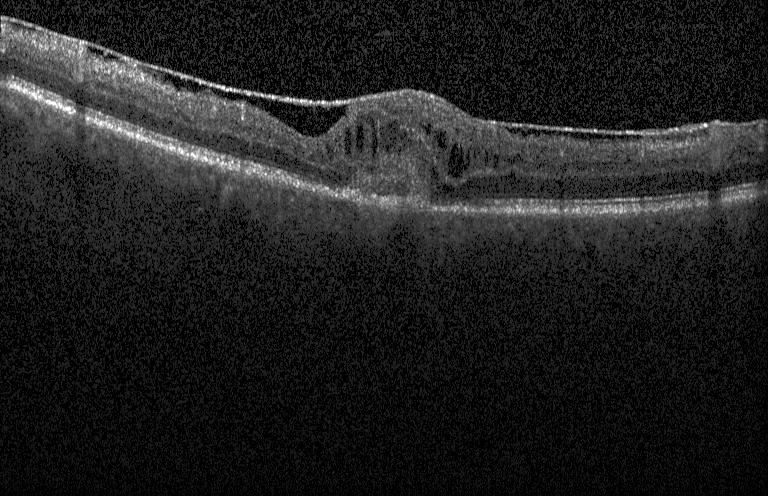 Macular scan; retinal OCT cross-section — This B-scan demonstrates choroidal neovascularization.